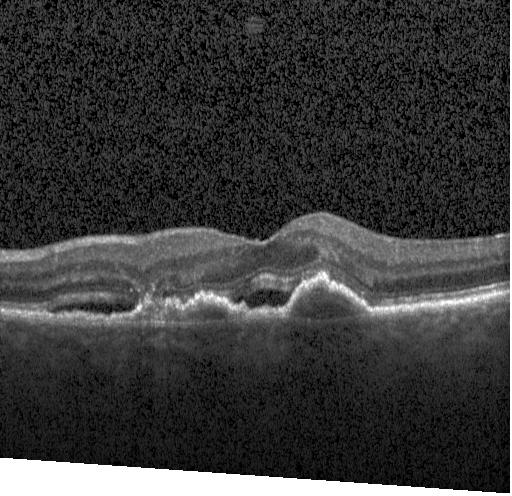

The scan shows choroidal neovascularization (CNV).